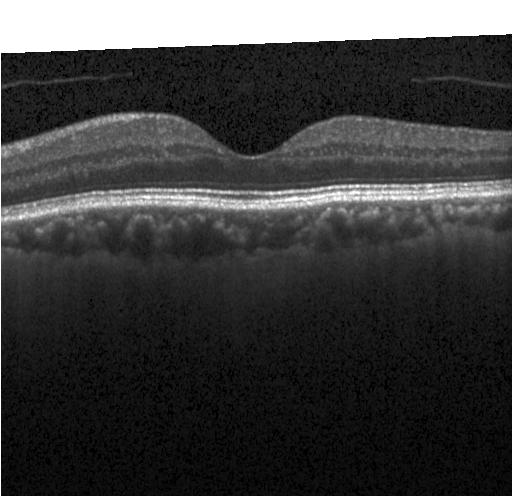

Retinal OCT cross-section showing no choroidal neovascularization, diabetic macular edema, or drusen.